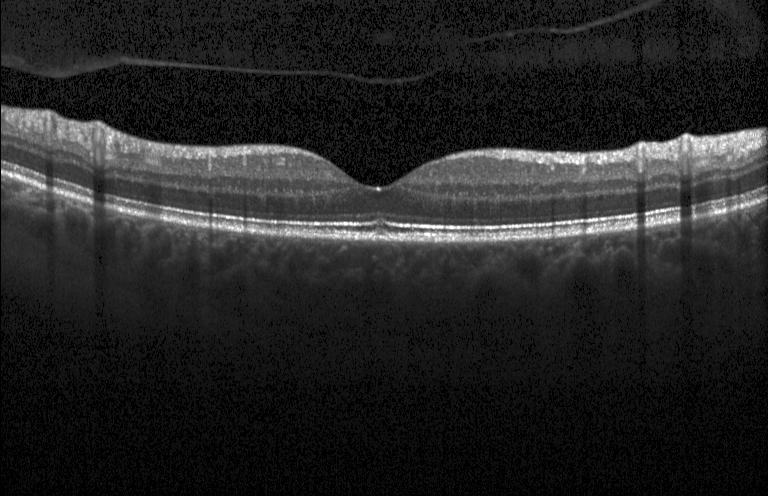

Finding: no evidence of CNV, DME, or drusen.